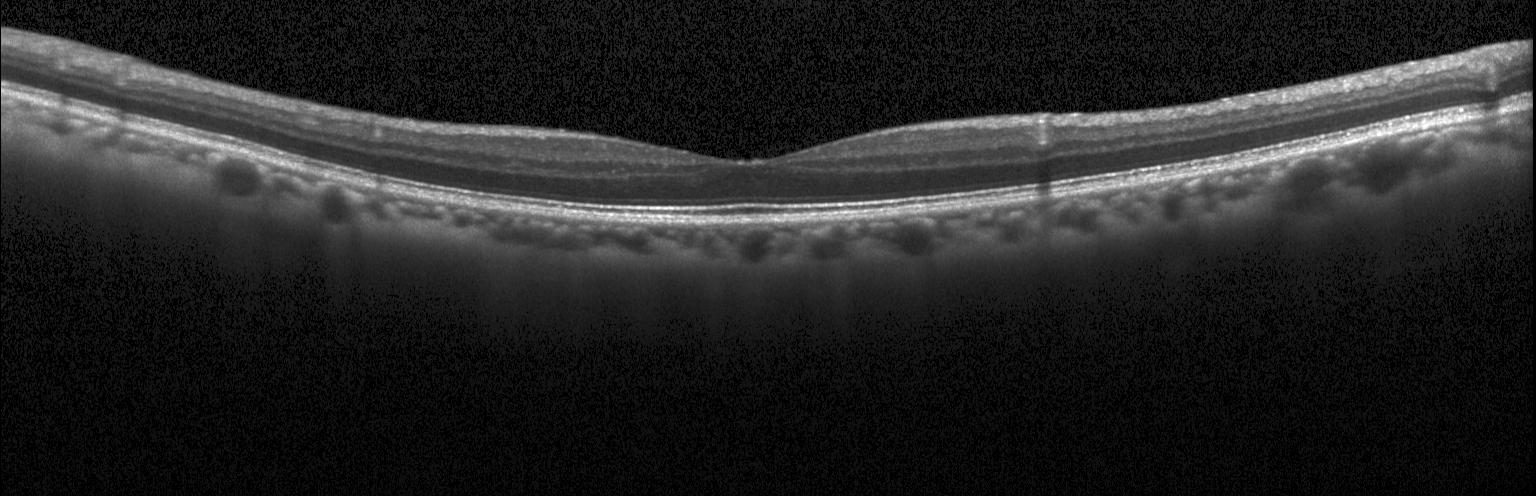 OCT scan showing no CNV, DME, or drusen.